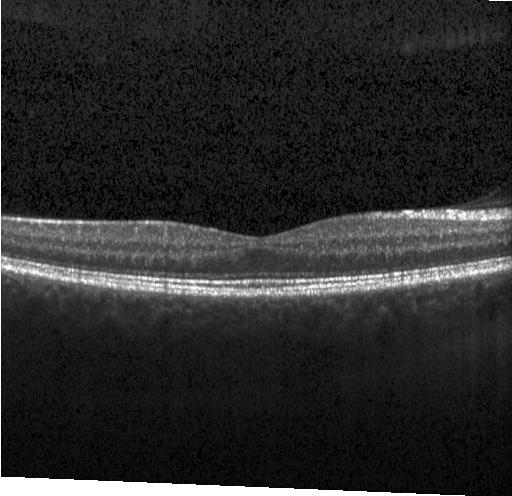

Impression: neither choroidal neovascularization, diabetic macular edema, nor drusen.